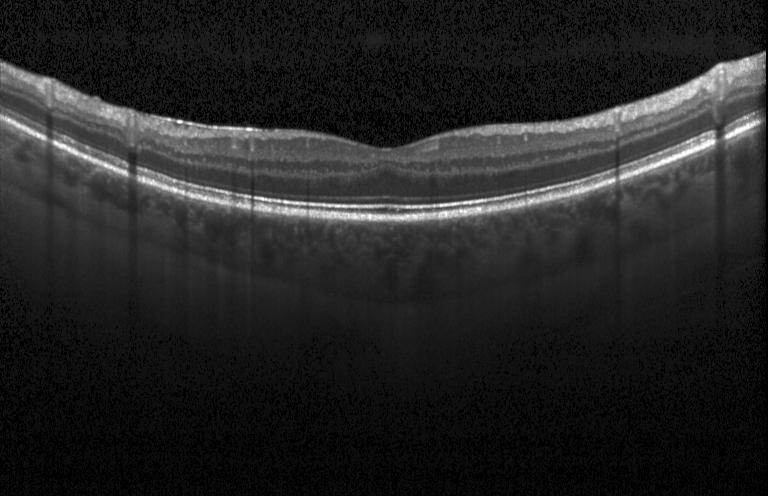
OCT scan showing no choroidal neovascularization, no diabetic macular edema, and no drusen.